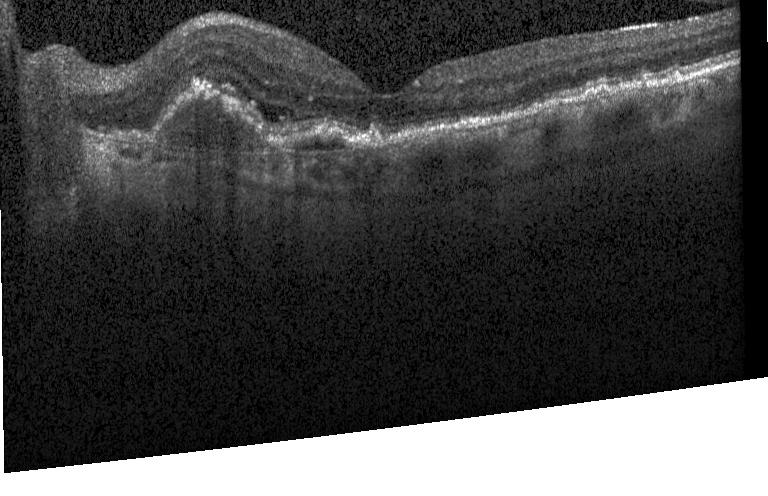

Spectral-domain optical coherence tomography; OCT B-scan; acquired on a Heidelberg Spectralis; fovea-centered
Finding: choroidal neovascularization (CNV).